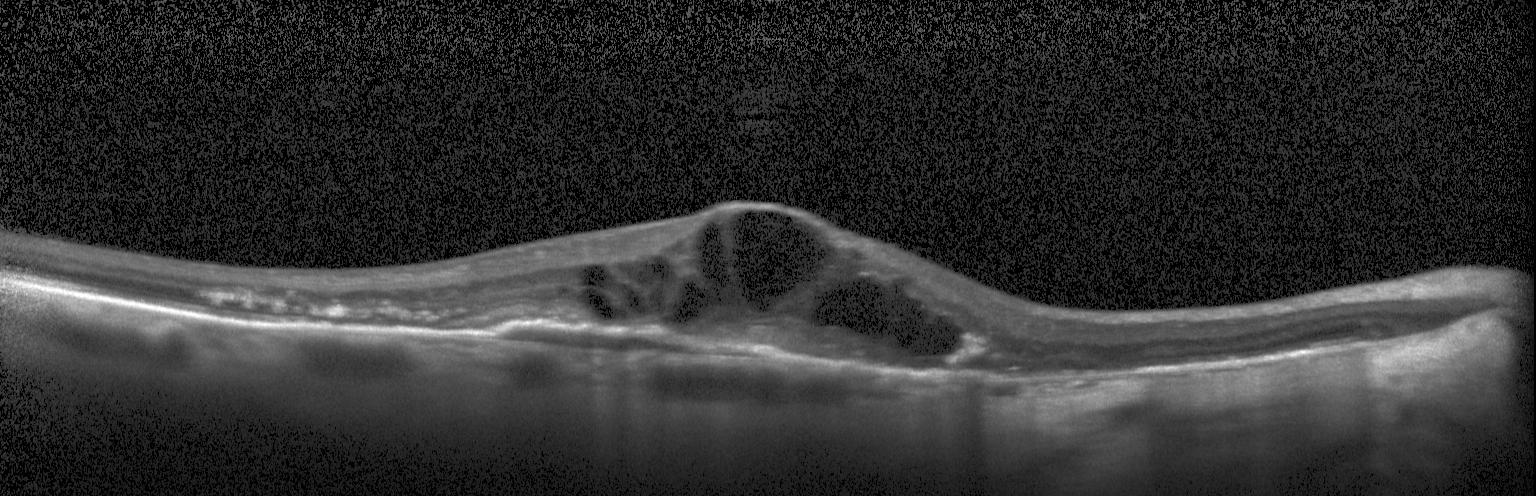 This B-scan demonstrates a choroidal neovascular membrane.